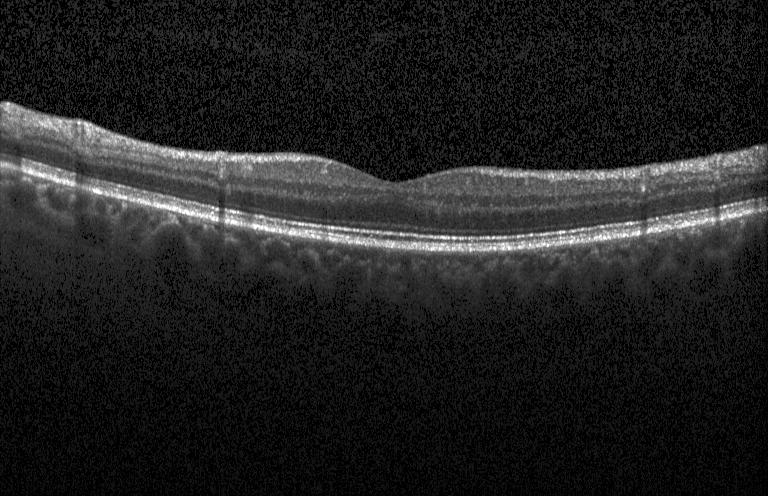 Spectral-domain optical coherence tomography · retinal OCT B-scan · Heidelberg Spectralis OCT system. Diagnosis: no evidence of choroidal neovascularization, diabetic macular edema, or drusen.